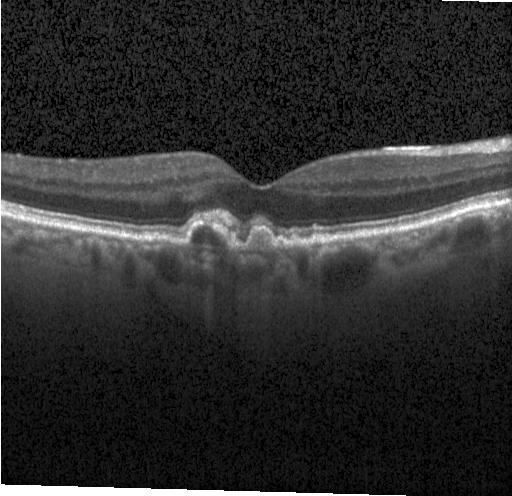 Instrument: Heidelberg Spectralis · optical coherence tomography B-scan · spectral-domain OCT. Impression: choroidal neovascularization (CNV).